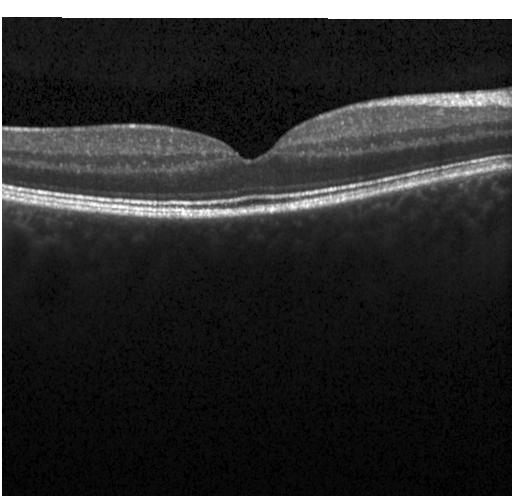 Retinal OCT cross-section. Diagnosis: no evidence of choroidal neovascularization, diabetic macular edema, or drusen.